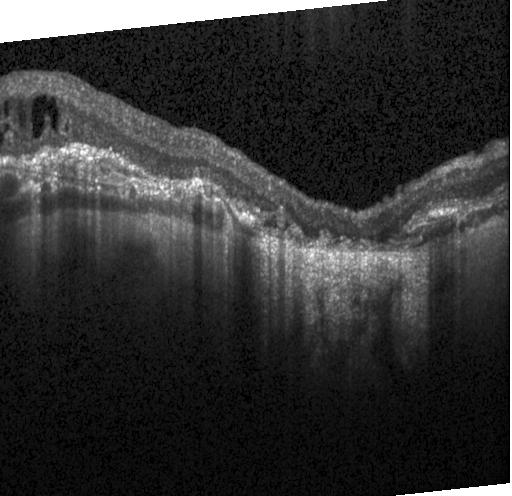

This B-scan demonstrates a choroidal neovascular membrane.